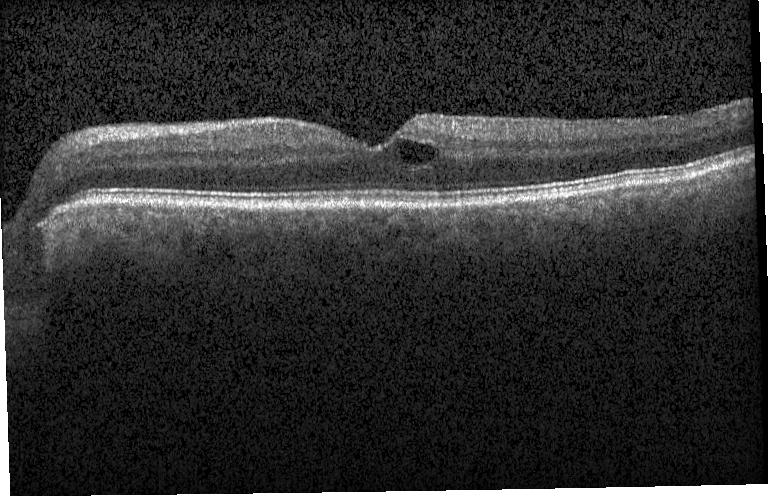 Macular OCT demonstrating diabetic macular edema.